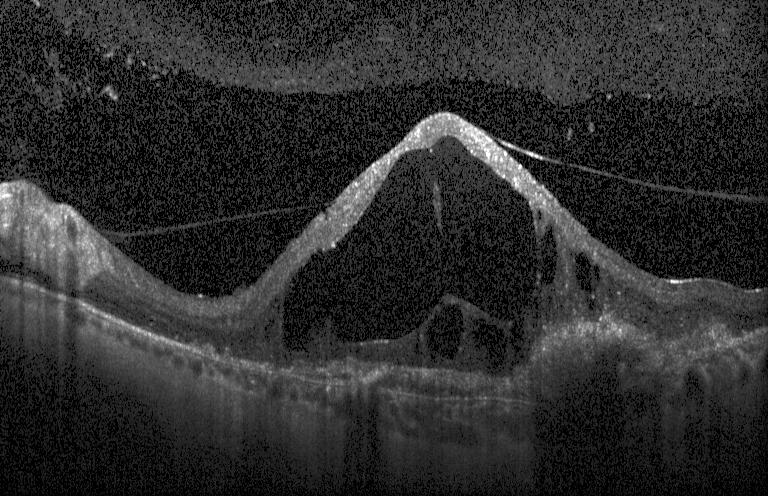 The scan shows a choroidal neovascular membrane.